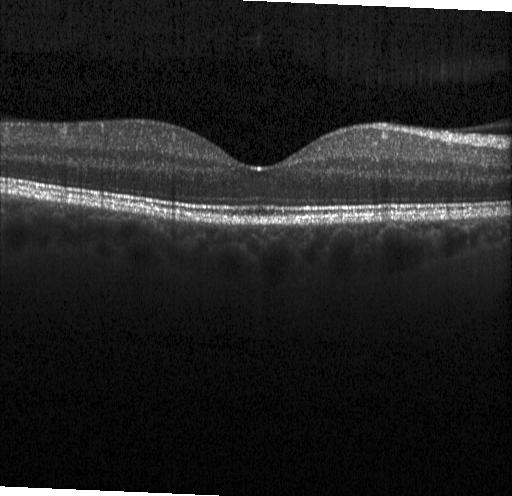 Optical coherence tomography B-scan · SD-OCT — Impression: no choroidal neovascularization, no diabetic macular edema, and no drusen.